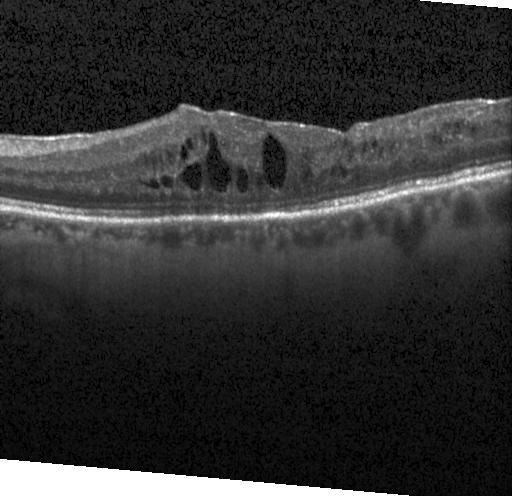 Spectral-domain OCT · OCT B-scan.
The scan shows diabetic macular edema.